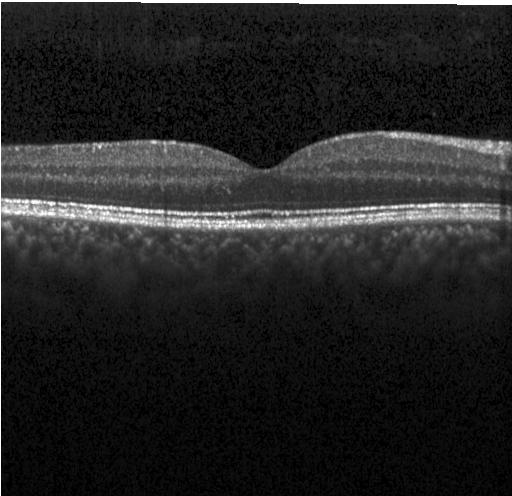
Acquired on a Heidelberg Spectralis · OCT line scan. Macular OCT: neither choroidal neovascularization, diabetic macular edema, nor drusen.